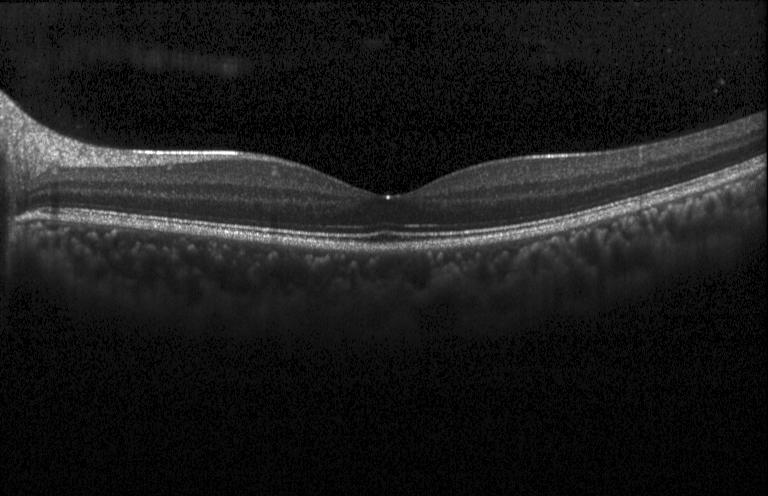
Retinal OCT cross-section — No CNV, DME, or drusen.